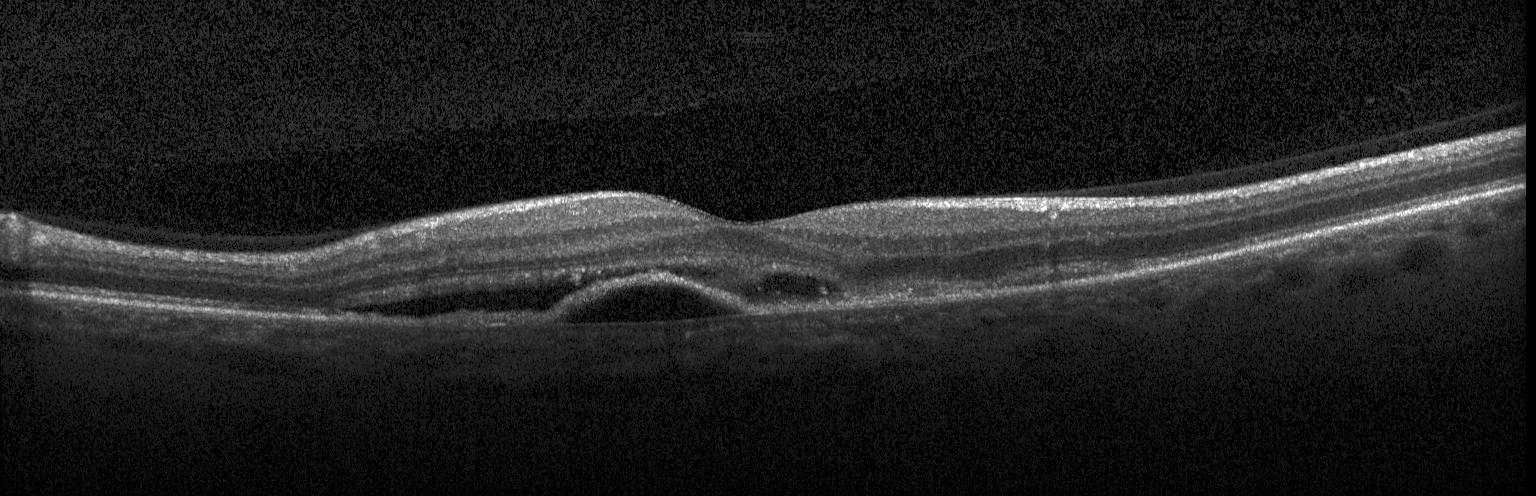
Through the macula · spectral-domain optical coherence tomography · retinal OCT cross-section · acquired on a Heidelberg Spectralis
Assessment: a choroidal neovascular membrane.